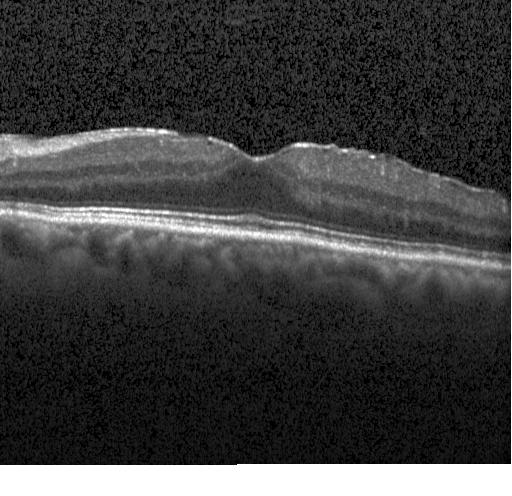

Impression: neither CNV, DME, nor drusen.